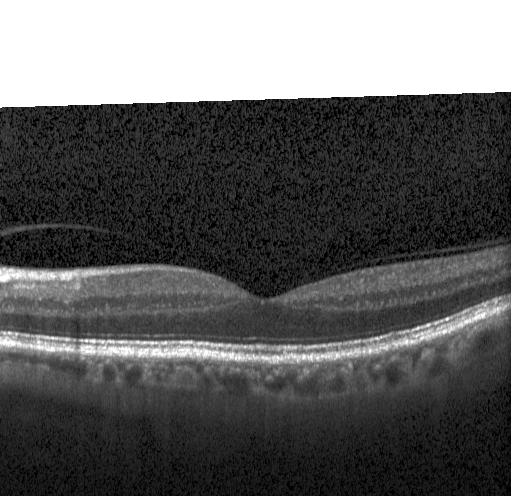
Retinal OCT cross-section showing no choroidal neovascularization, no diabetic macular edema, and no drusen.